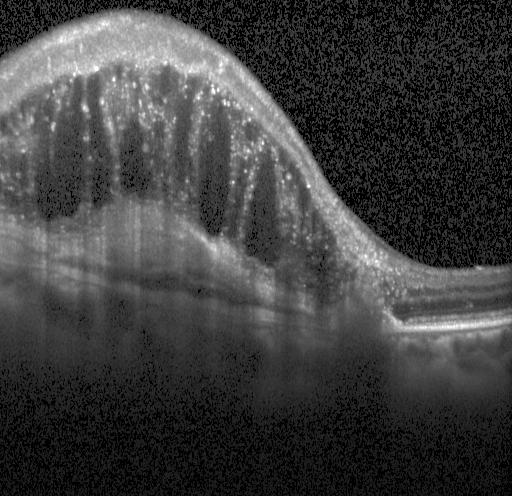
Assessment: diabetic macular edema (DME).